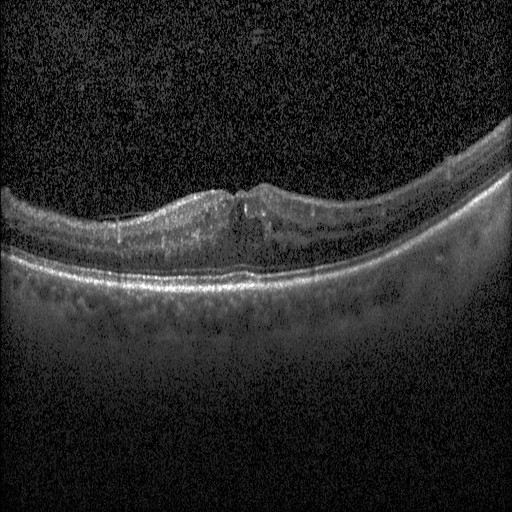
SD-OCT, instrument: Heidelberg Spectralis, through the macula, OCT B-scan. Macular OCT: diabetic macular edema (DME).